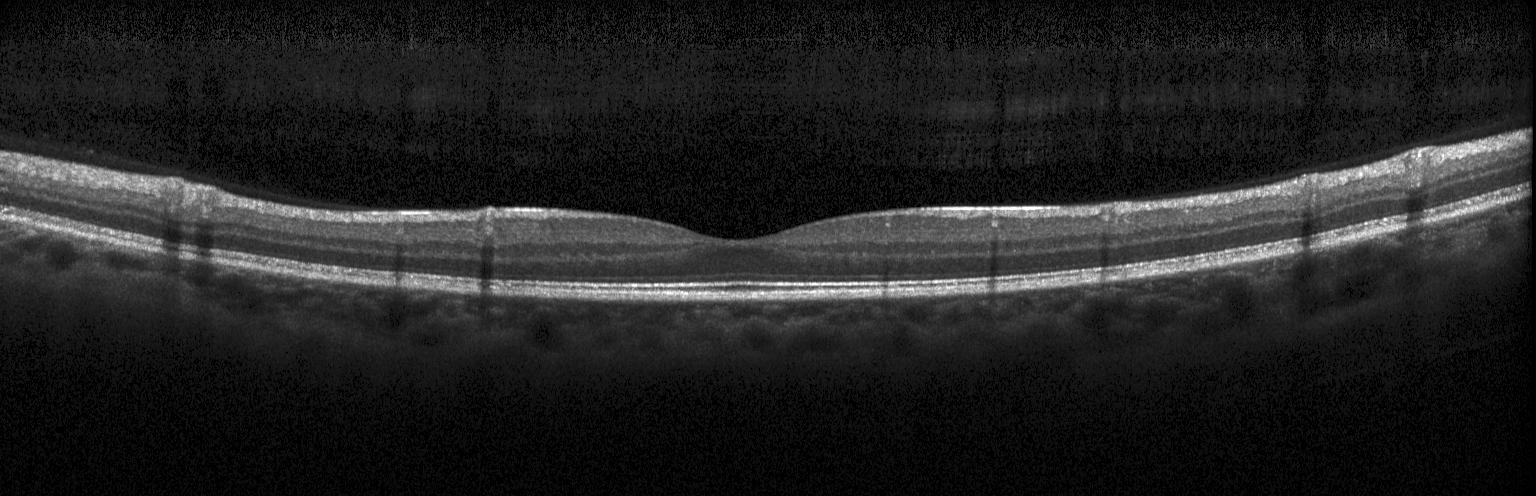

Finding: no CNV, DME, or drusen.